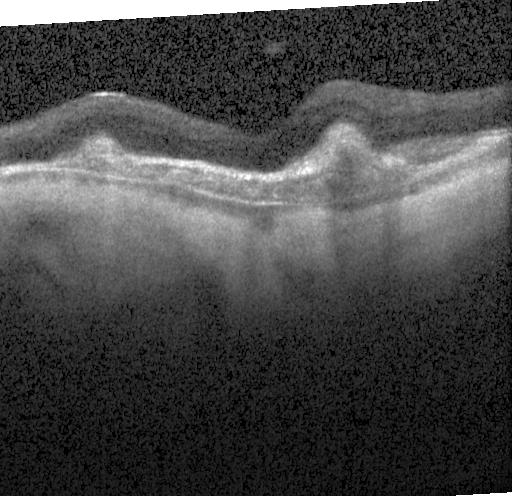 Retinal OCT cross-section. Diagnosis: choroidal neovascularization (CNV).